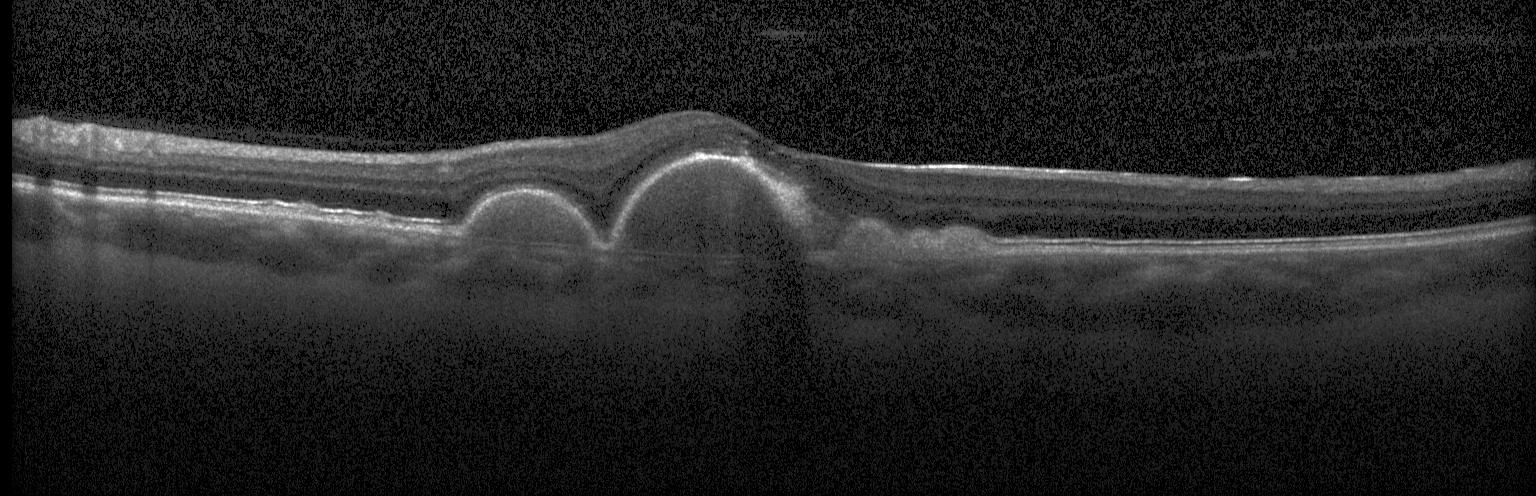

Retinal OCT B-scan; horizontal scan through the fovea
Dx: CNV.